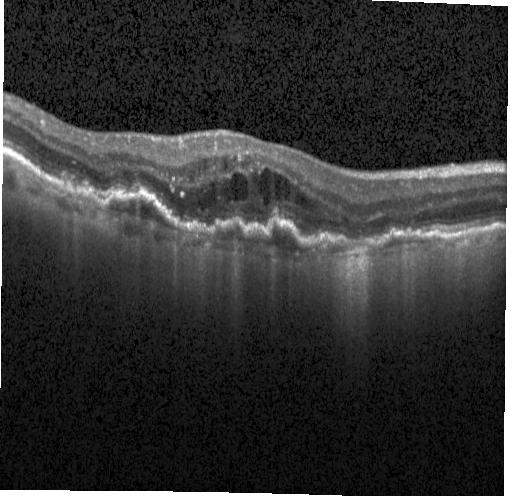 OCT scan showing a choroidal neovascular membrane.